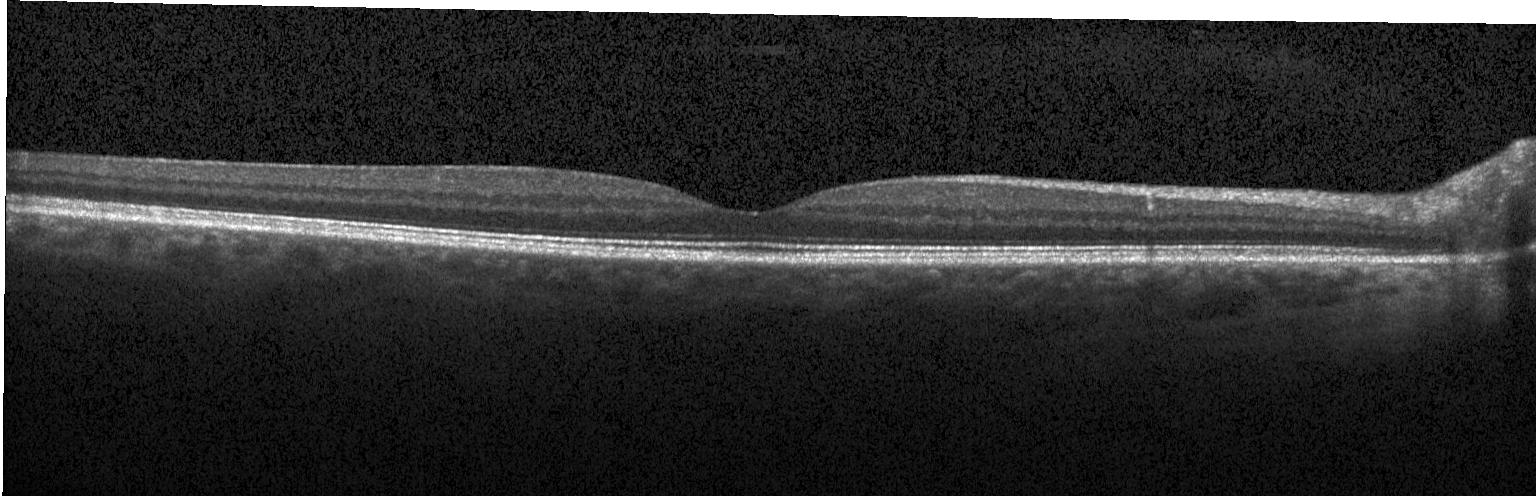
Macular scan. Acquired on a Heidelberg Spectralis. Spectral-domain OCT. Retinal OCT B-scan
This B-scan demonstrates no CNV, no DME, and no drusen.